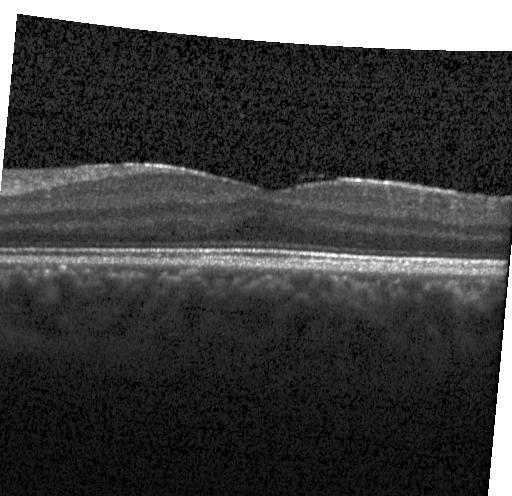

Retinal OCT B-scan.
No choroidal neovascularization, diabetic macular edema, or drusen.